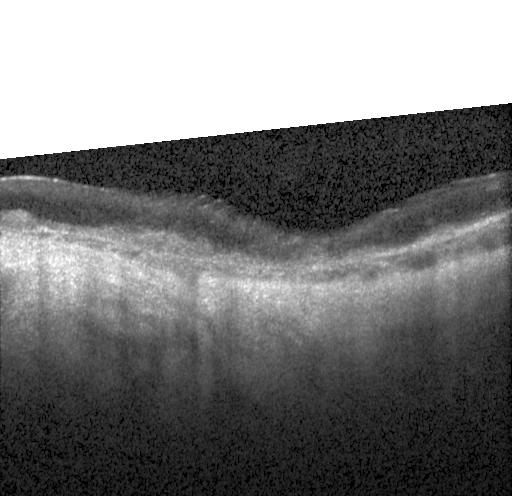

OCT B-scan · macular scan · SD-OCT.
The scan shows CNV.